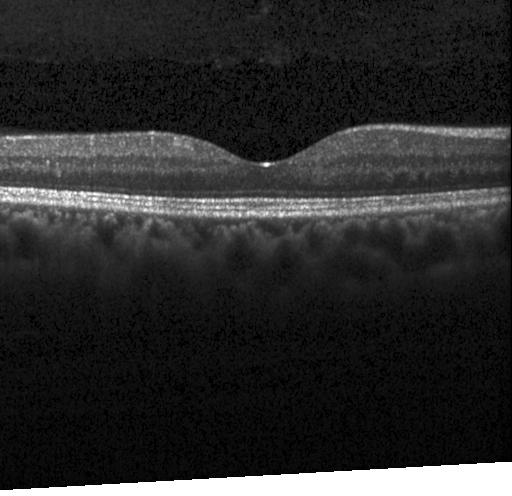 Horizontal scan through the fovea. Spectral-domain OCT. Retinal OCT B-scan. Heidelberg Spectralis. No choroidal neovascularization, diabetic macular edema, or drusen.